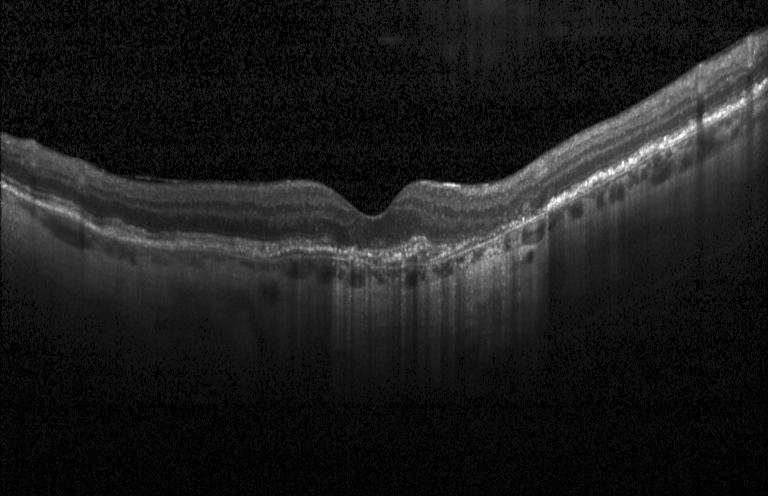
Optical coherence tomography scan — Impression: CNV.